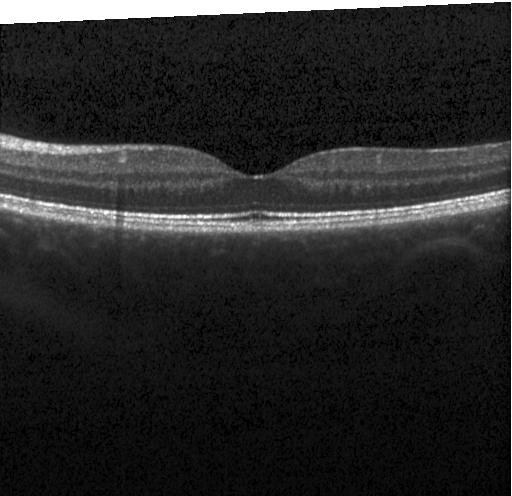
Dx: neither CNV, DME, nor drusen.